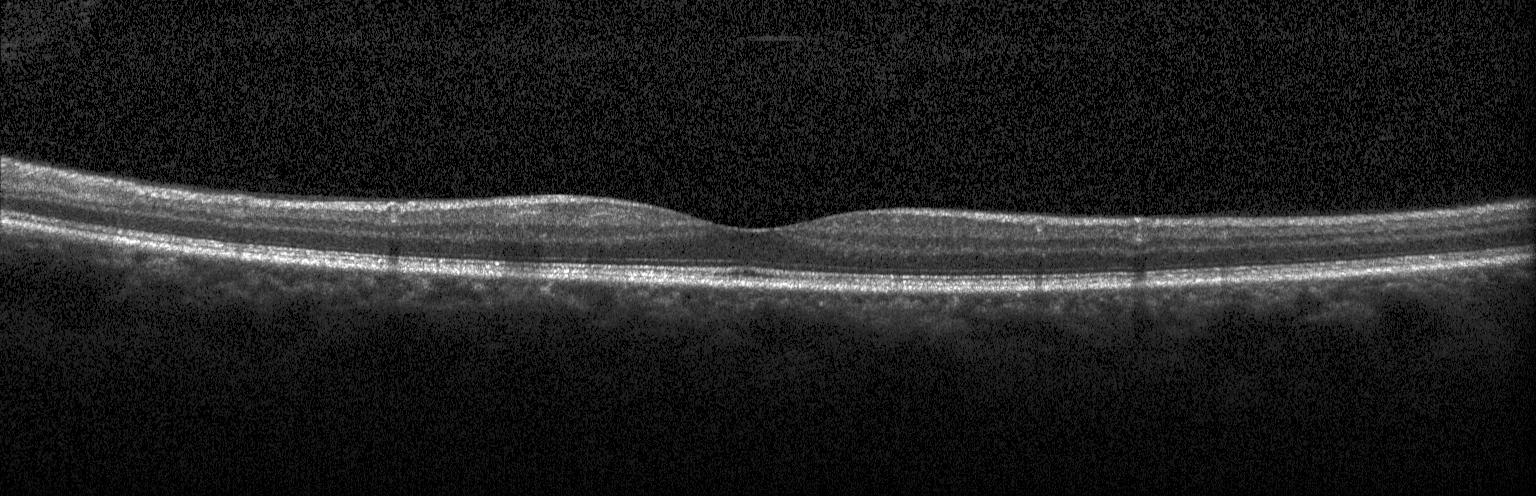
Diagnosis: neither choroidal neovascularization, diabetic macular edema, nor drusen.